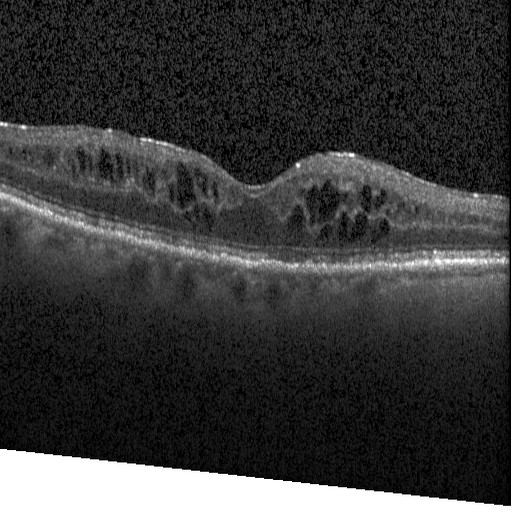 DME.